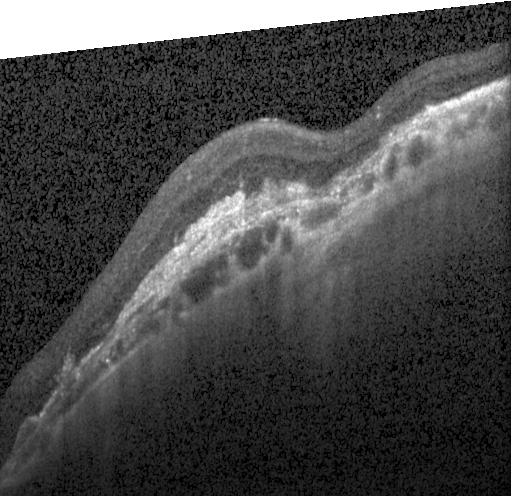

Diagnosis: a choroidal neovascular membrane.